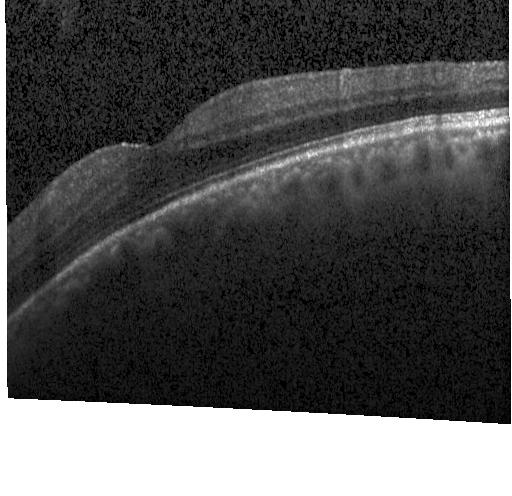

Optical coherence tomography scan. Fovea-centered. Macular OCT: neither choroidal neovascularization, diabetic macular edema, nor drusen.